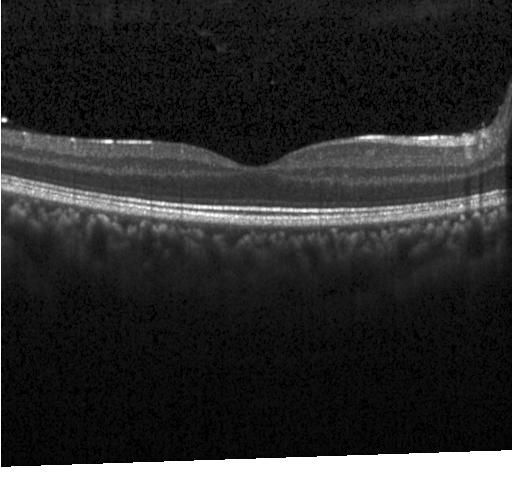 Through the macula · Heidelberg Spectralis OCT system · spectral-domain OCT · retinal OCT B-scan
Impression: no evidence of choroidal neovascularization, diabetic macular edema, or drusen.